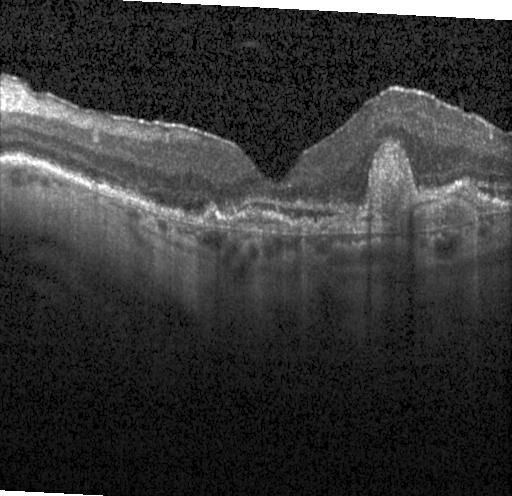

Macular OCT: choroidal neovascularization.